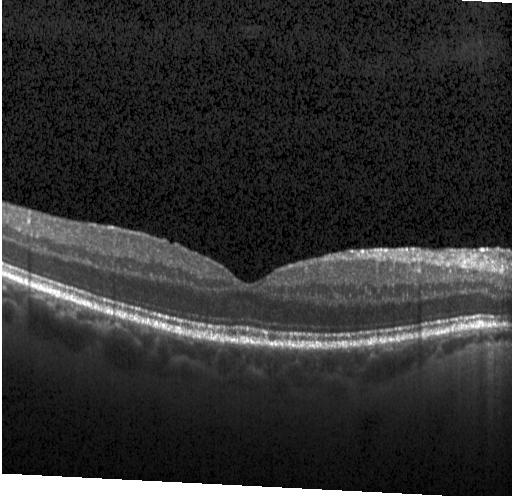 OCT B-scan showing neither choroidal neovascularization, diabetic macular edema, nor drusen.